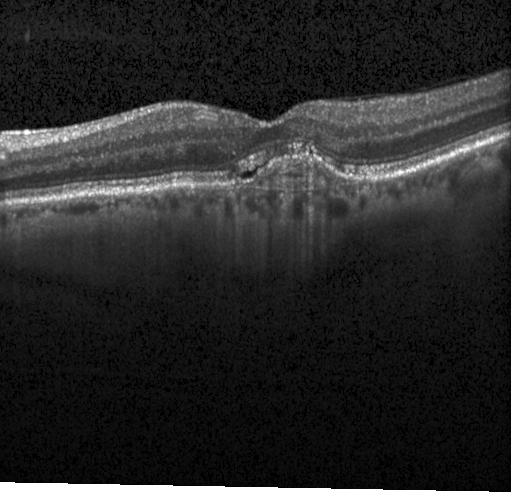
Retinal OCT B-scan. SD-OCT.
OCT finding: choroidal neovascularization.